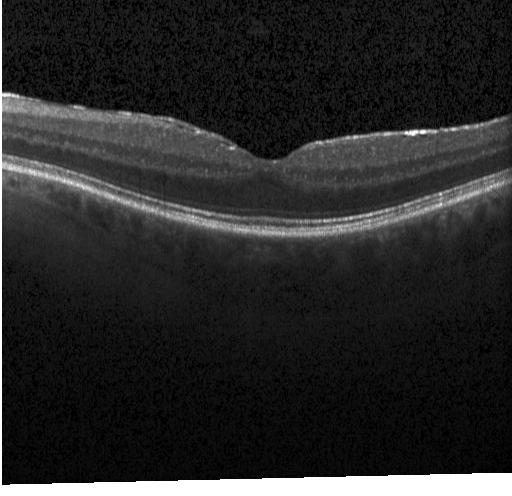

Spectral-domain optical coherence tomography · fovea-centered · OCT B-scan · Heidelberg Spectralis OCT system — OCT finding: no choroidal neovascularization, no diabetic macular edema, and no drusen.